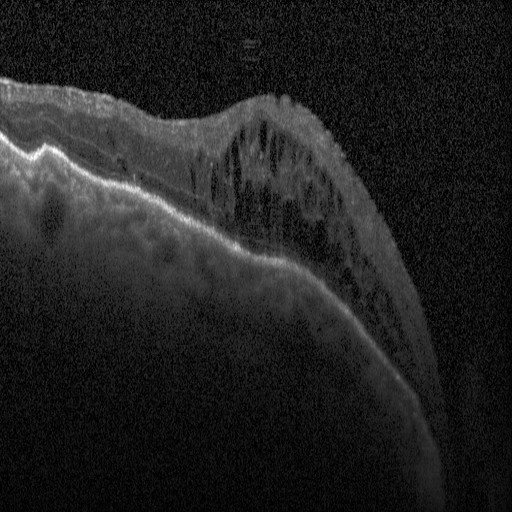
Spectral-domain optical coherence tomography, Heidelberg Spectralis, macular scan, retinal OCT B-scan. Impression: diabetic macular edema (DME).